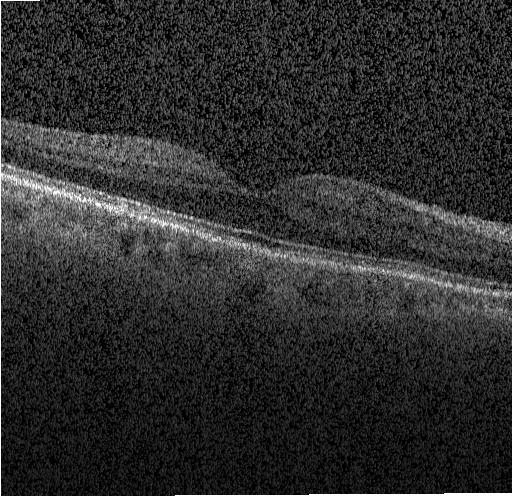 Retinal OCT B-scan; acquired on a Heidelberg Spectralis
No CNV, DME, or drusen.